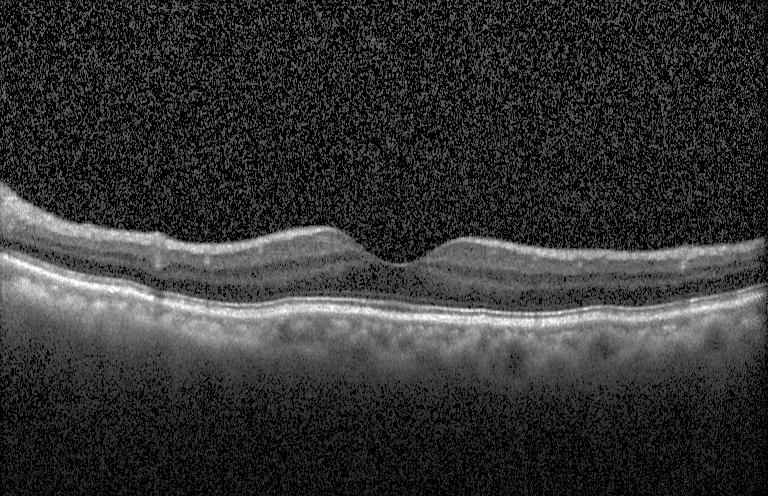 Finding: no evidence of choroidal neovascularization, diabetic macular edema, or drusen.